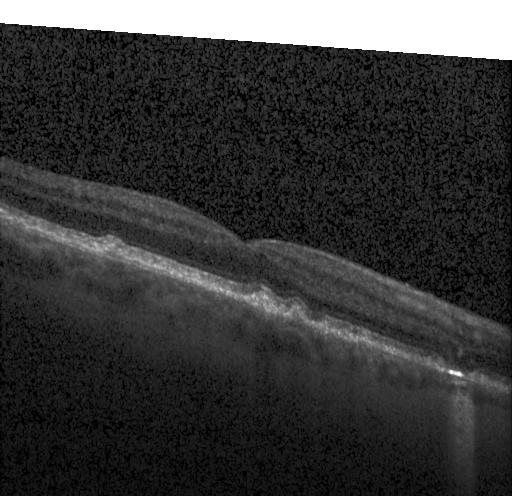
Optical coherence tomography scan — Diagnosis: multiple drusen.